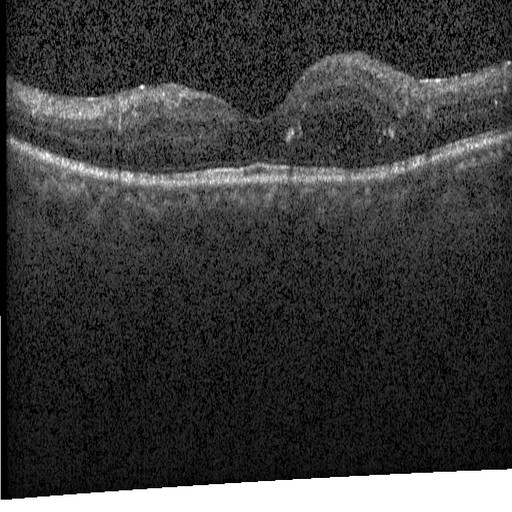
Optical coherence tomography B-scan — Finding: diabetic macular edema (DME).